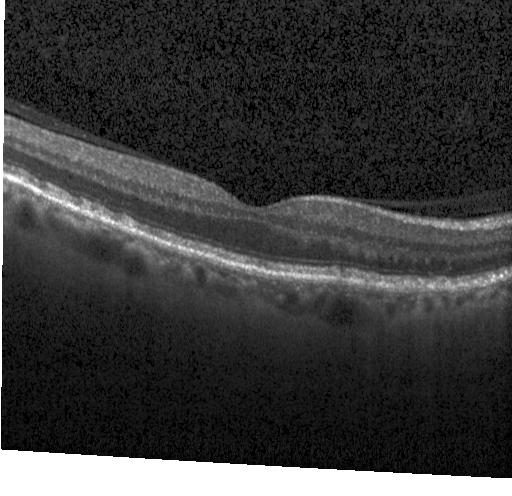 OCT scan showing no choroidal neovascularization, no diabetic macular edema, and no drusen.